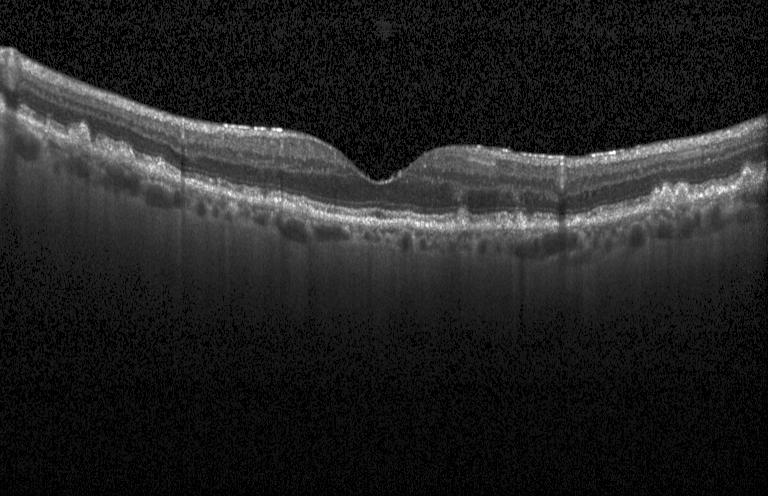 Acquired on a Heidelberg Spectralis; OCT B-scan; spectral-domain OCT.
Multiple drusen.